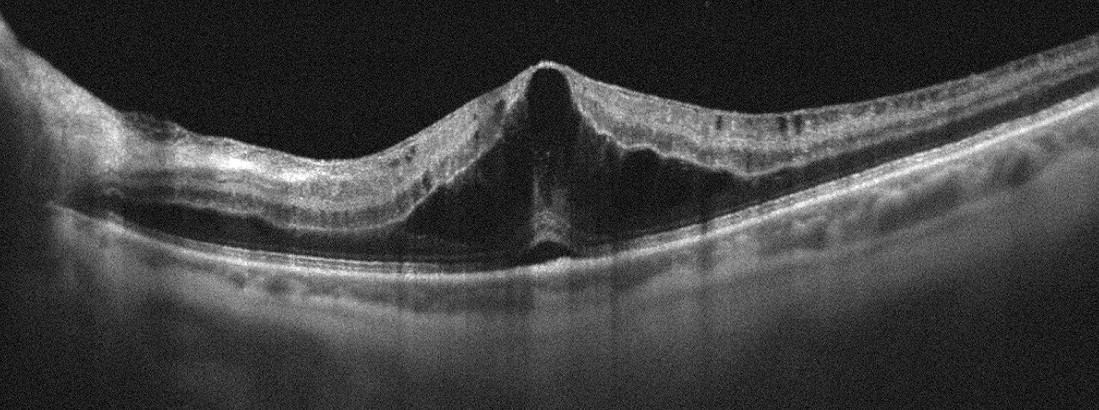

Retinal OCT cross-section showing retinal vein occlusion.